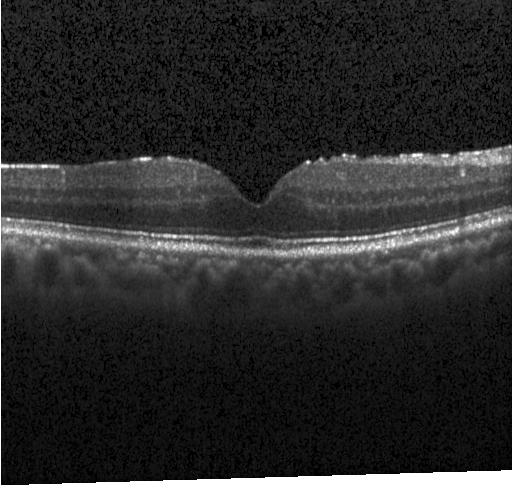

Spectral-domain OCT; fovea-centered; optical coherence tomography scan.
Diagnosis: no CNV, no DME, and no drusen.